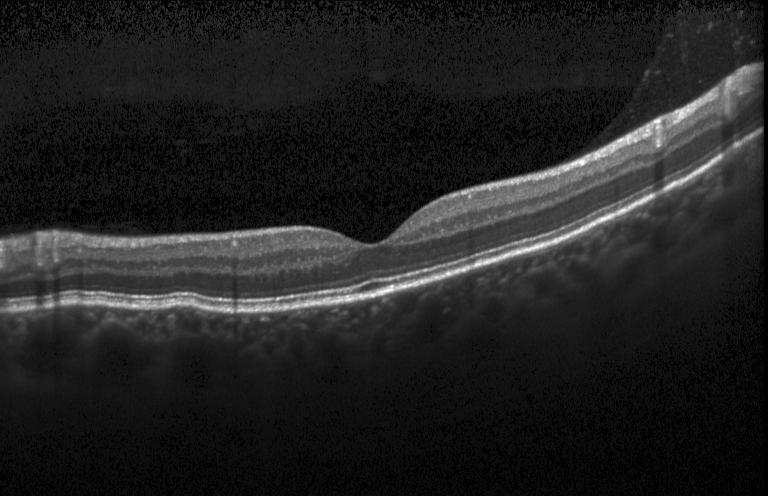 SD-OCT. Horizontal scan through the fovea. OCT line scan. Finding: neither choroidal neovascularization, diabetic macular edema, nor drusen.